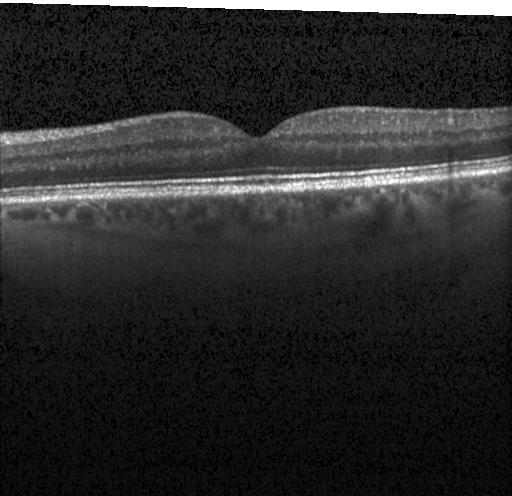
Optical coherence tomography B-scan — Assessment: no evidence of CNV, DME, or drusen.